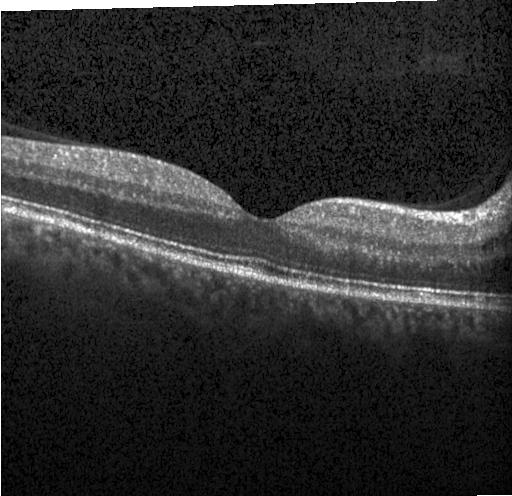
Finding: no choroidal neovascularization, no diabetic macular edema, and no drusen.